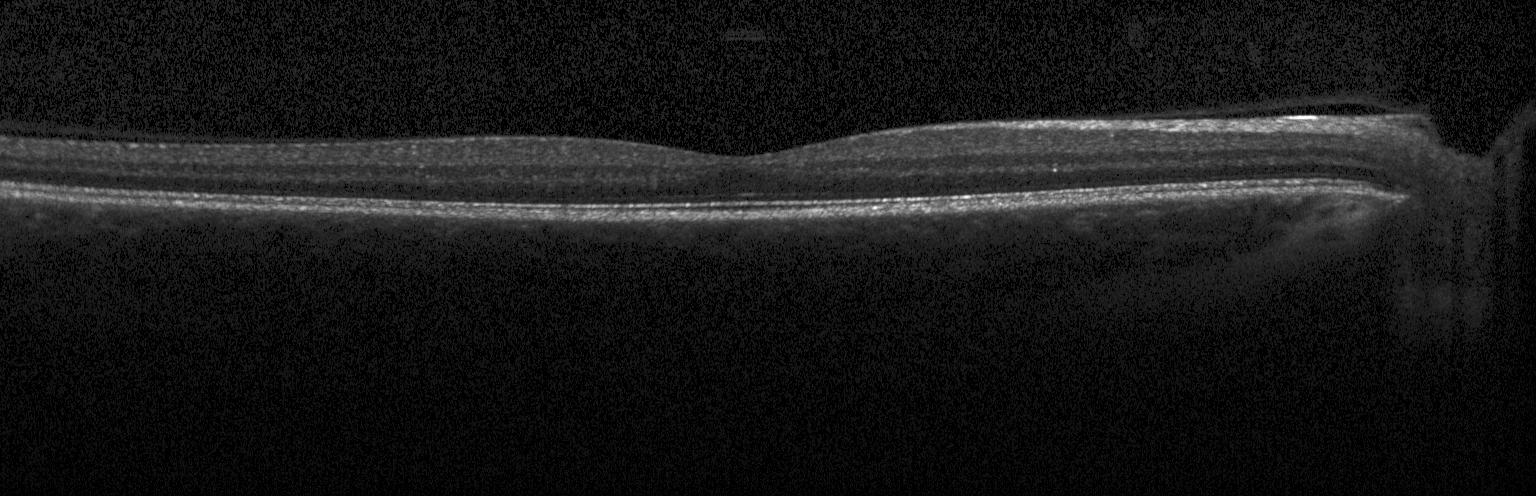
Finding: neither CNV, DME, nor drusen.